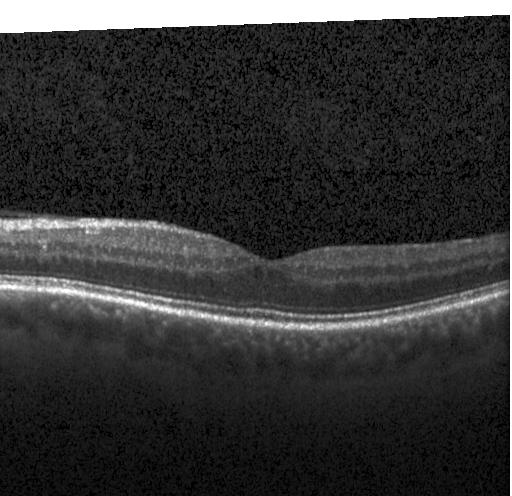 Diagnosis: no choroidal neovascularization, diabetic macular edema, or drusen.